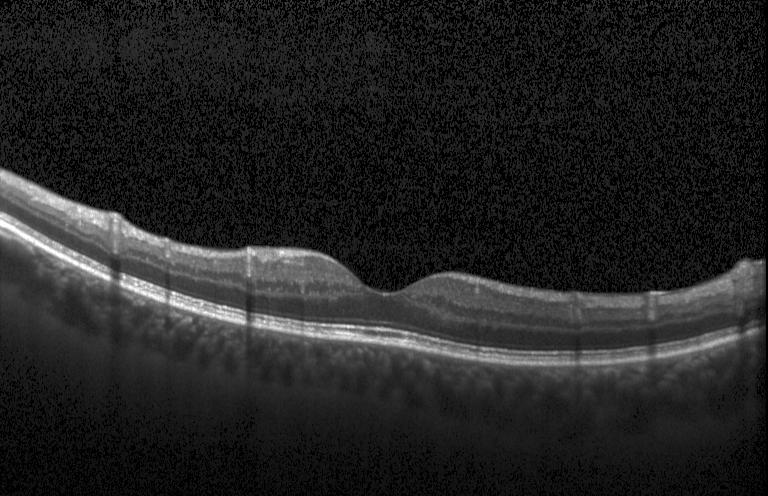

Optical coherence tomography scan · acquired on a Heidelberg Spectralis
No choroidal neovascularization, diabetic macular edema, or drusen.